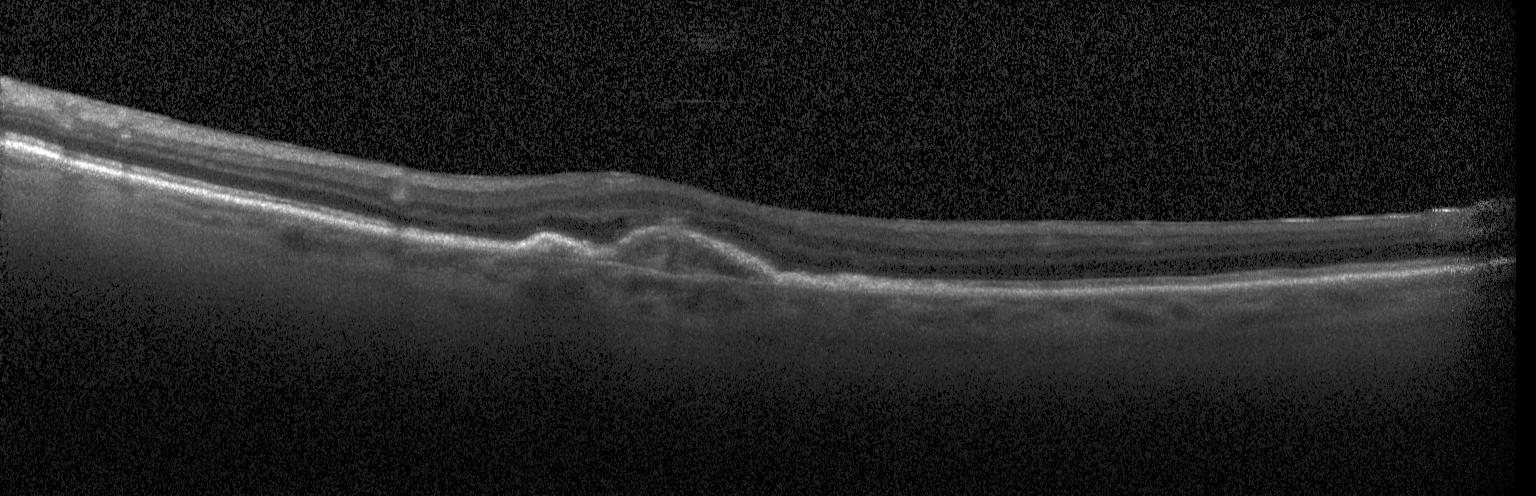
Retinal OCT B-scan.
This B-scan demonstrates a choroidal neovascular membrane.